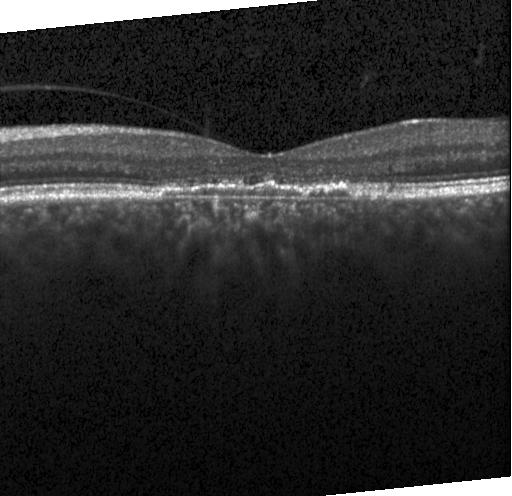

Retinal OCT B-scan — Finding: CNV.